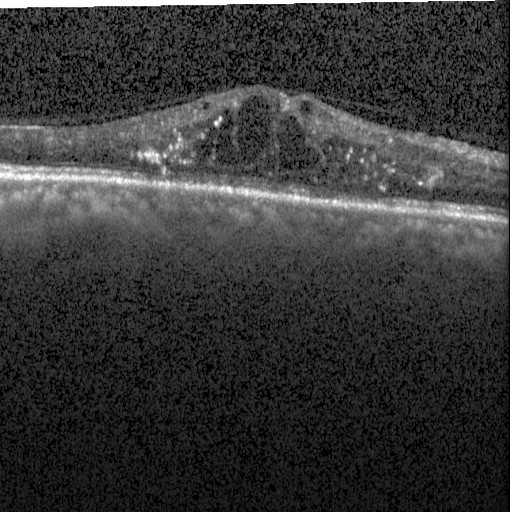

OCT scan showing diabetic macular edema.